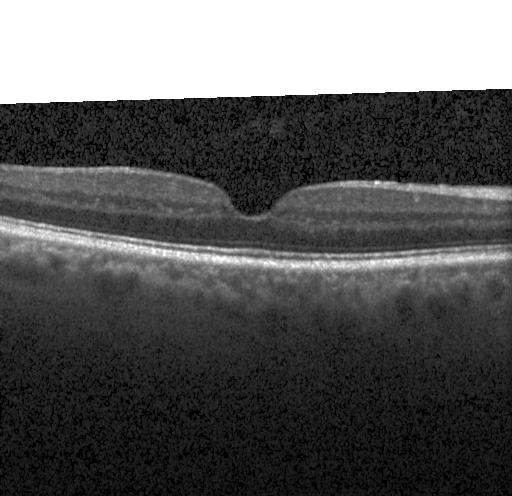
Retinal OCT cross-section. Impression: neither CNV, DME, nor drusen.